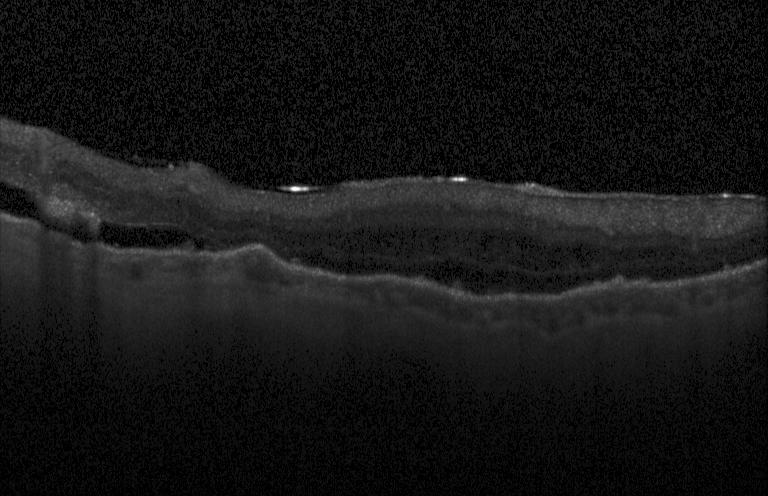
Dx: CNV.